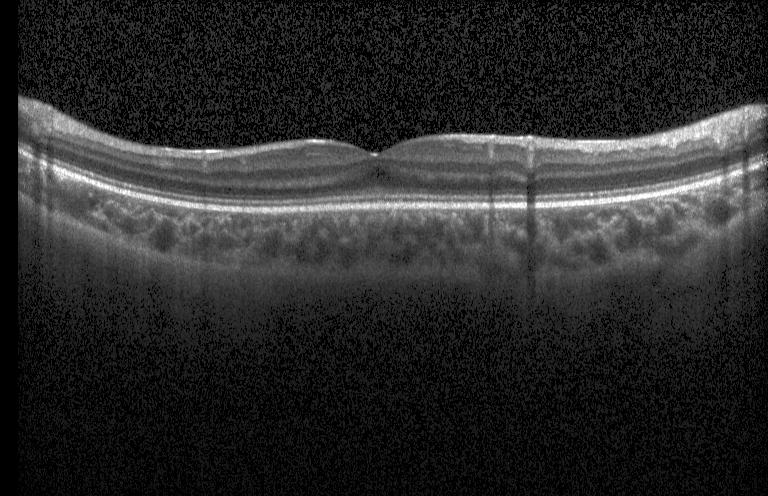 Retinal OCT cross-section showing no evidence of choroidal neovascularization, diabetic macular edema, or drusen.